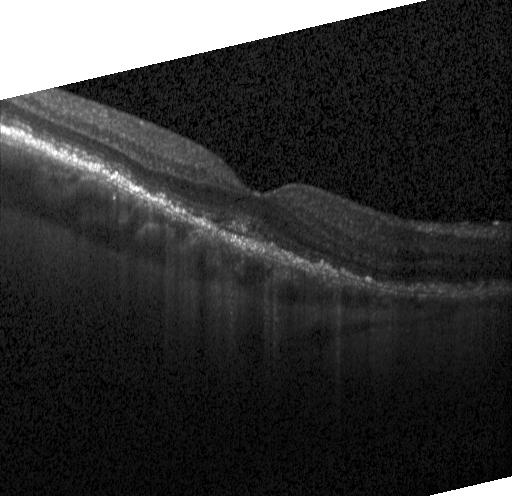 Macular OCT: CNV.